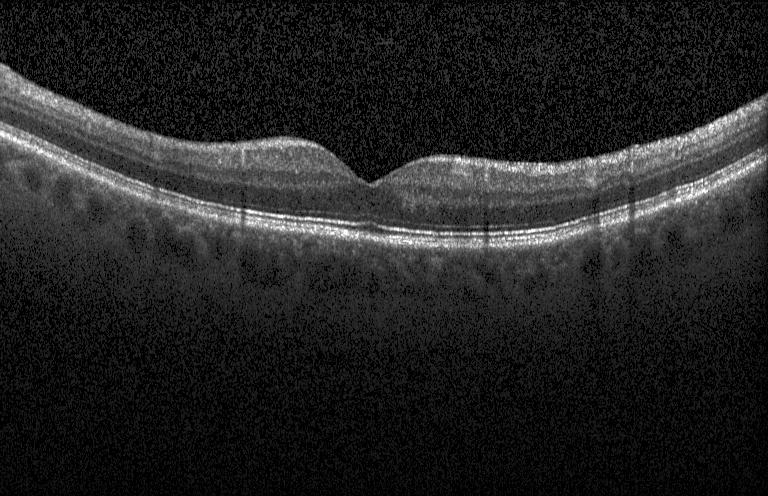 Macular scan · spectral-domain OCT · instrument: Heidelberg Spectralis · OCT B-scan
Diagnosis: no evidence of choroidal neovascularization, diabetic macular edema, or drusen.